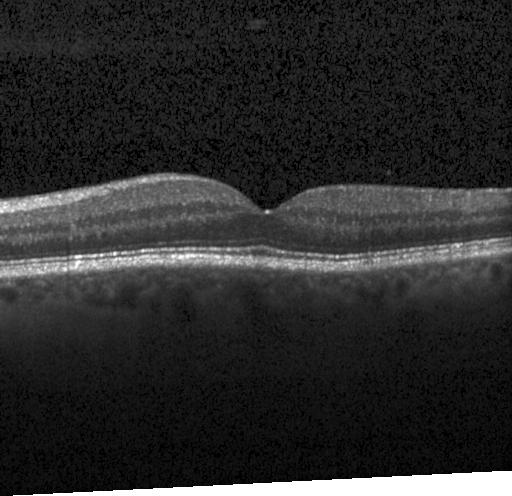

Impression: no CNV, DME, or drusen.